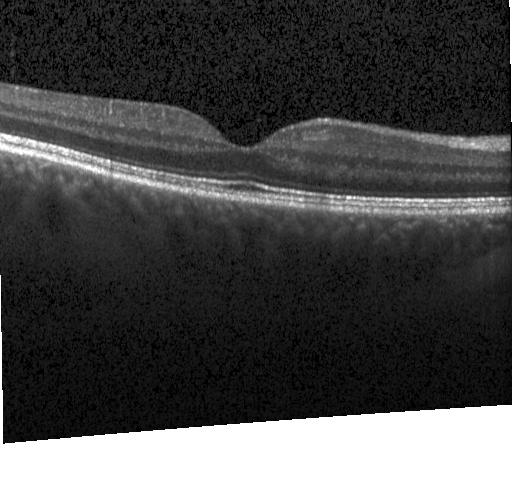
Retinal OCT cross-section; spectral-domain OCT; Heidelberg Spectralis OCT system; fovea-centered — Impression: no choroidal neovascularization, no diabetic macular edema, and no drusen.